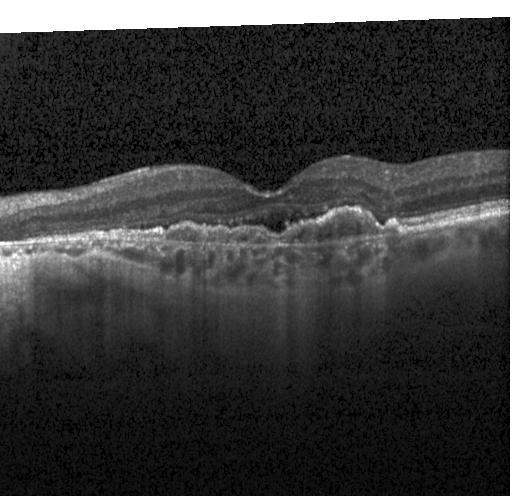
Acquired on a Heidelberg Spectralis. OCT line scan.
Diagnosis: a choroidal neovascular membrane.